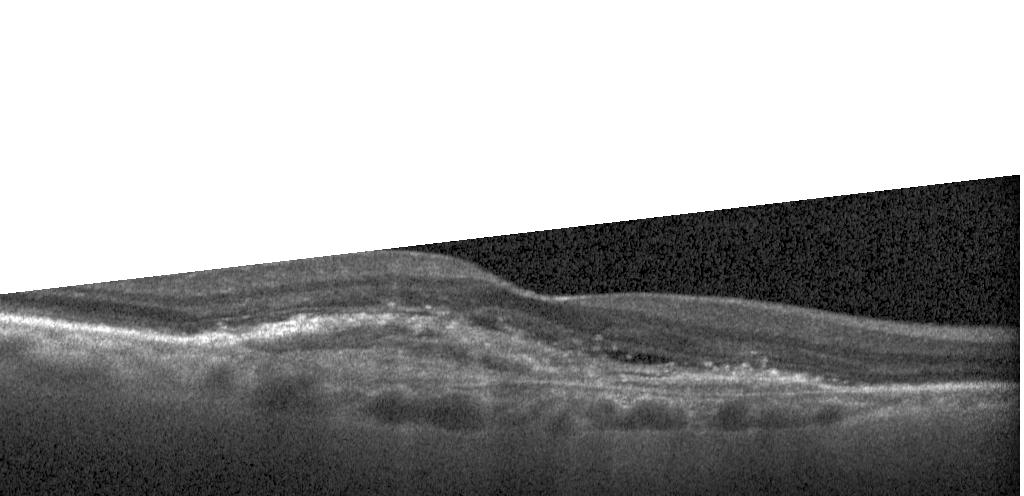

Spectral-domain OCT B-scan: a choroidal neovascular membrane.